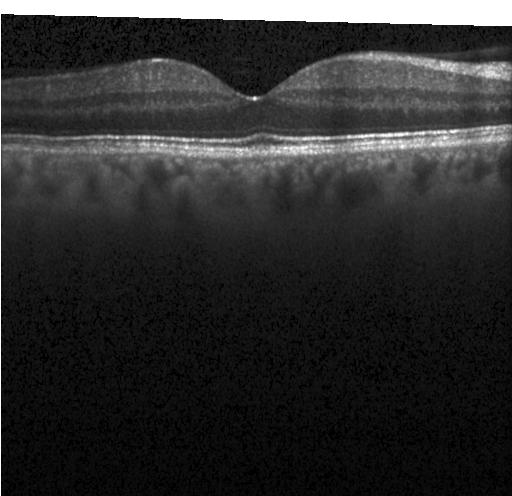
OCT finding: no choroidal neovascularization, diabetic macular edema, or drusen.